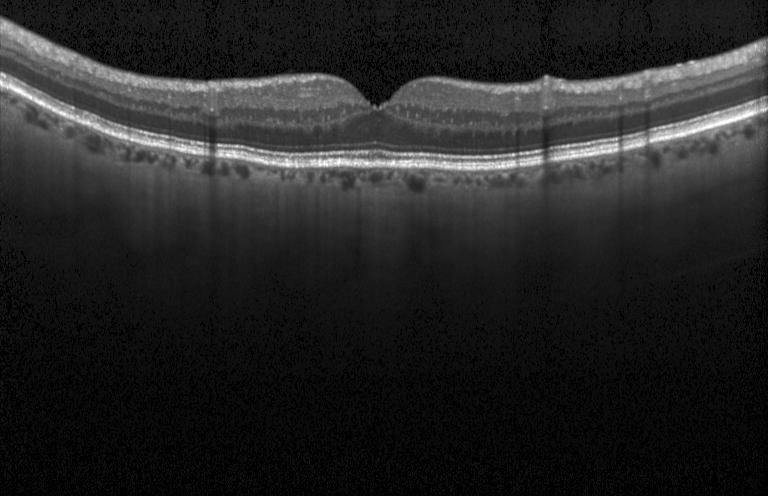

OCT B-scan showing no evidence of choroidal neovascularization, diabetic macular edema, or drusen.